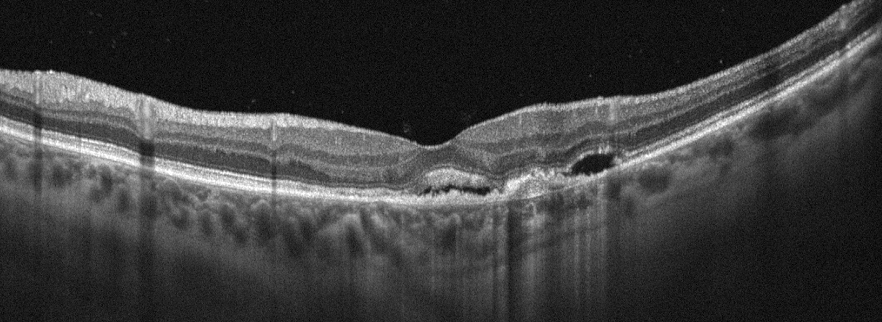 OCT B-scan, oculus sinister. Finding: age-related macular degeneration (AMD).